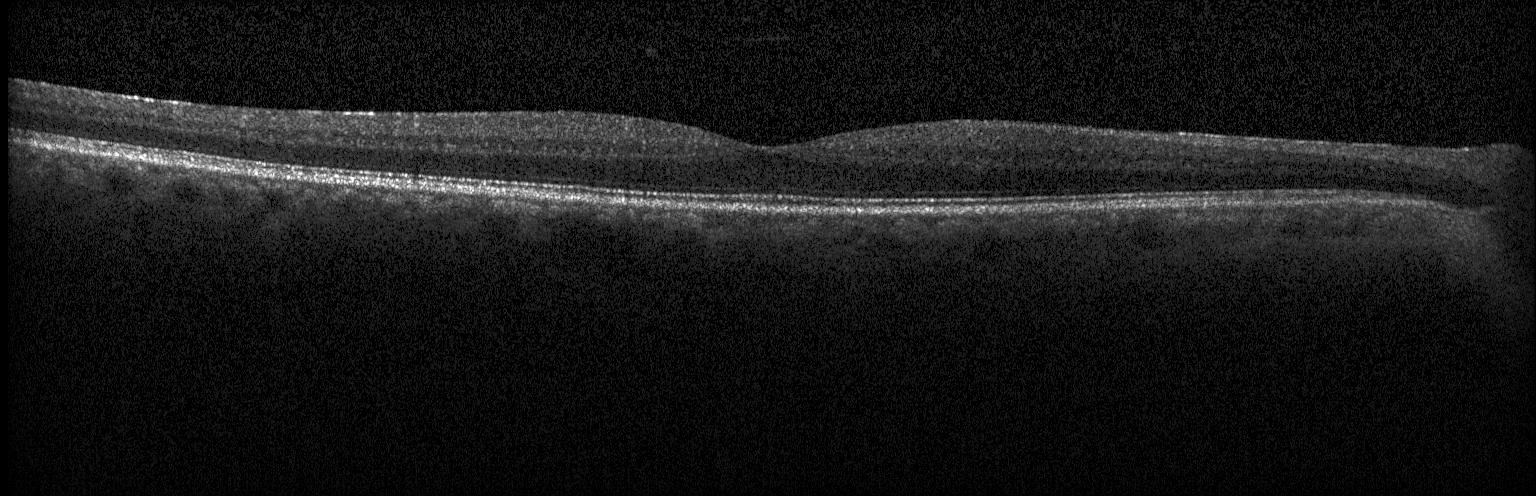 Heidelberg Spectralis; fovea-centered; OCT line scan. Impression: no choroidal neovascularization, no diabetic macular edema, and no drusen.